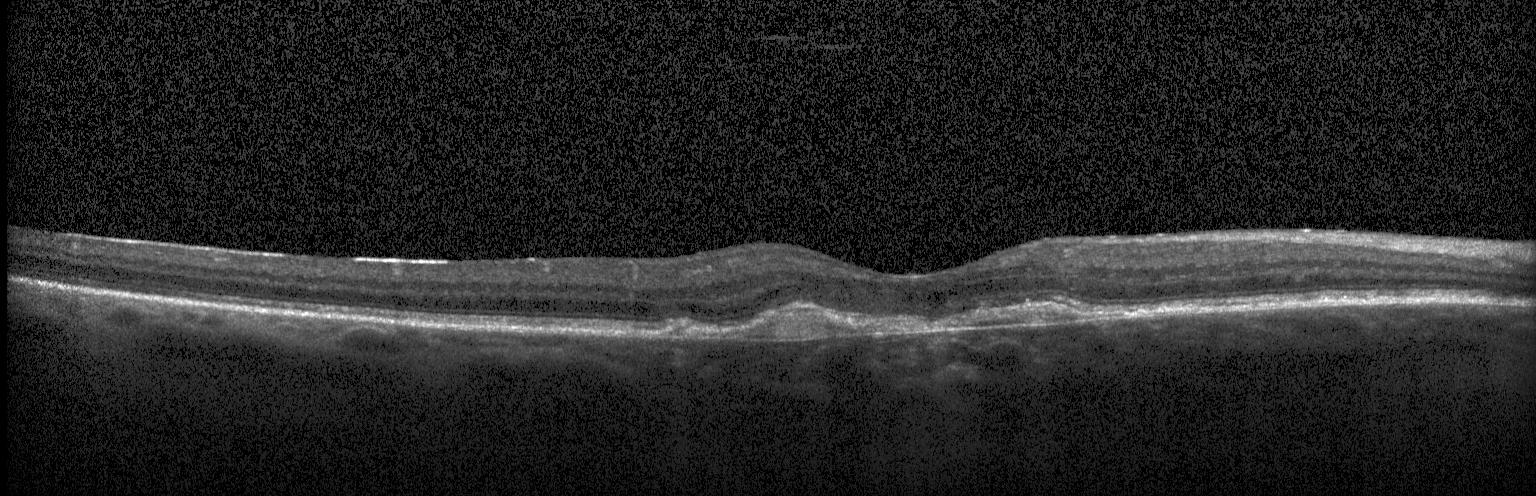

The scan shows CNV.